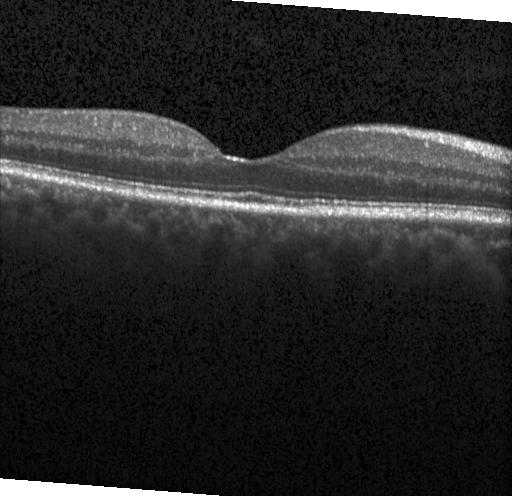 Optical coherence tomography B-scan · spectral-domain OCT · Heidelberg Spectralis OCT system · horizontal scan through the fovea.
Macular OCT: neither CNV, DME, nor drusen.